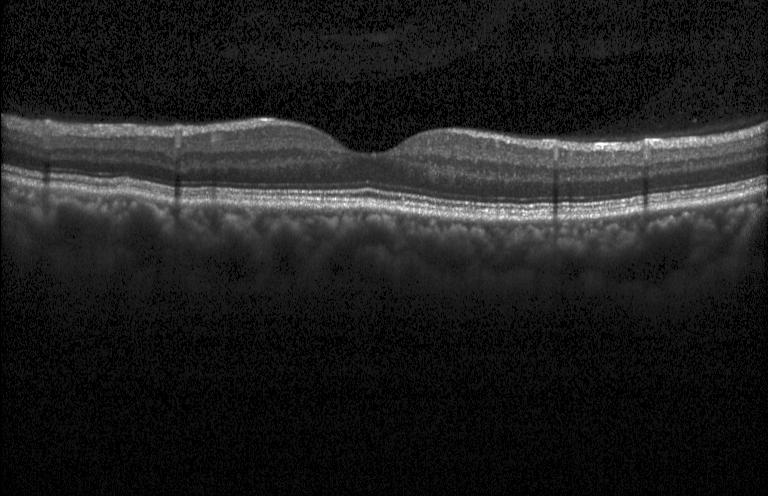
Instrument: Heidelberg Spectralis, spectral-domain OCT, optical coherence tomography scan, fovea-centered — Finding: no evidence of CNV, DME, or drusen.